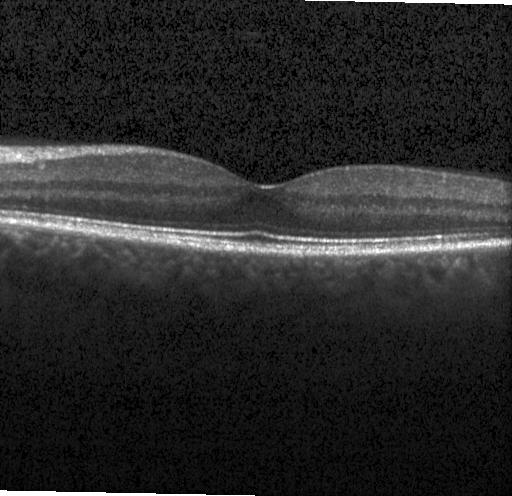 Optical coherence tomography scan. Neither choroidal neovascularization, diabetic macular edema, nor drusen.